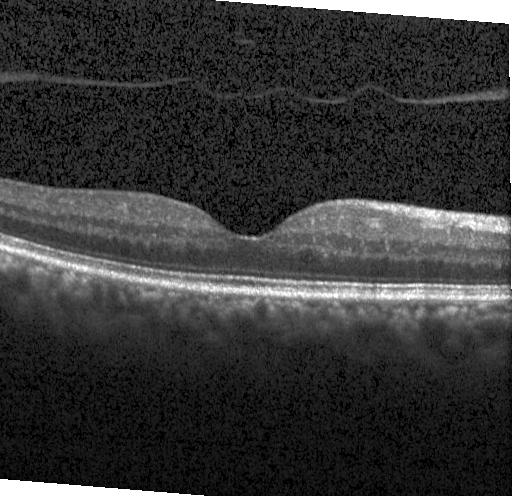

Optical coherence tomography B-scan; Heidelberg Spectralis. Diagnosis: no CNV, no DME, and no drusen.